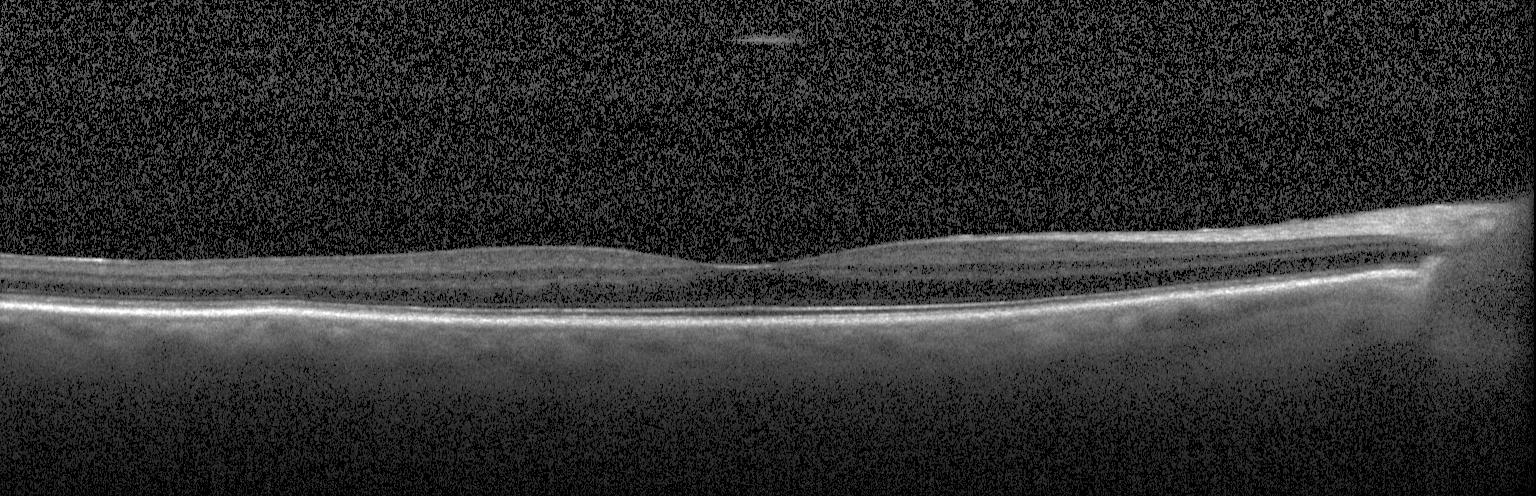

Through the macula, optical coherence tomography scan.
Dx: no choroidal neovascularization, diabetic macular edema, or drusen.